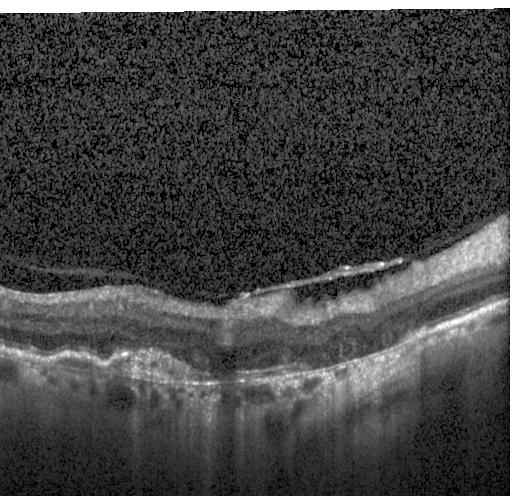 Retinal OCT cross-section. Spectral-domain OCT. Acquired on a Heidelberg Spectralis
Finding: a choroidal neovascular membrane.